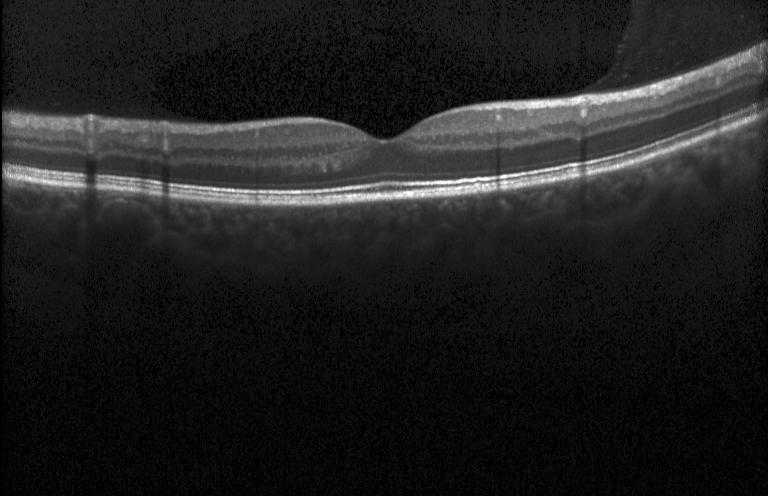 Instrument: Heidelberg Spectralis · centered on the fovea · optical coherence tomography B-scan. No choroidal neovascularization, no diabetic macular edema, and no drusen.